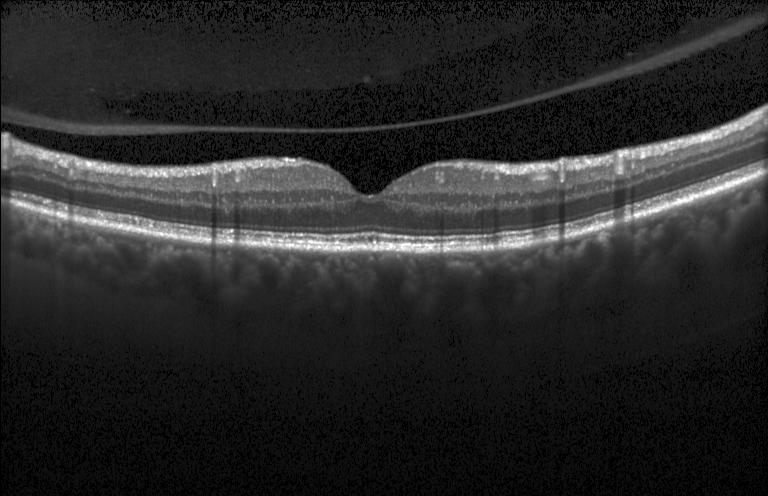

Impression: no evidence of choroidal neovascularization, diabetic macular edema, or drusen.